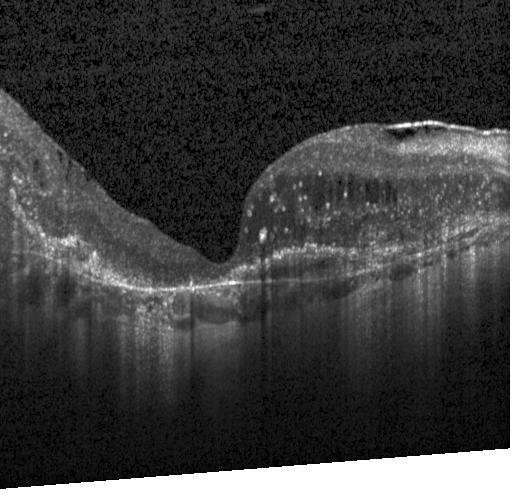
Retinal OCT cross-section showing a choroidal neovascular membrane.